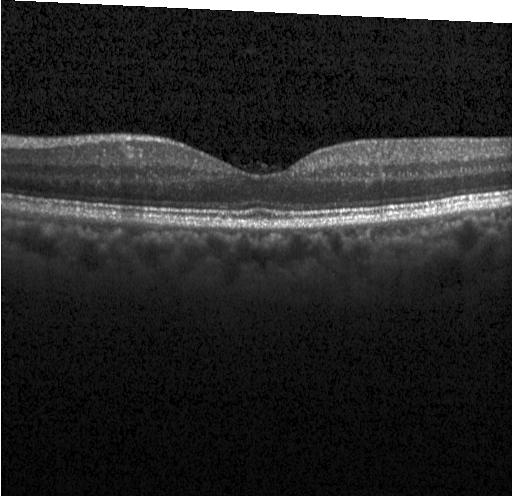
No choroidal neovascularization, no diabetic macular edema, and no drusen.